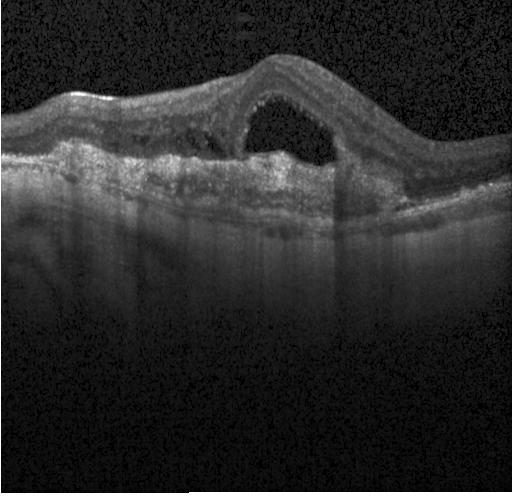

Spectral-domain OCT, centered on the fovea, optical coherence tomography B-scan — Dx: a choroidal neovascular membrane.